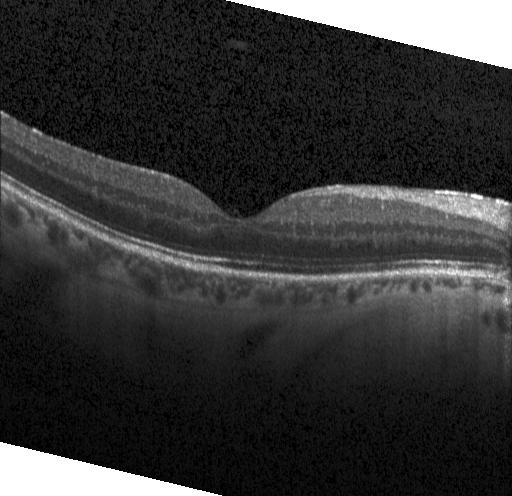

SD-OCT · OCT B-scan · macular scan. Finding: neither choroidal neovascularization, diabetic macular edema, nor drusen.